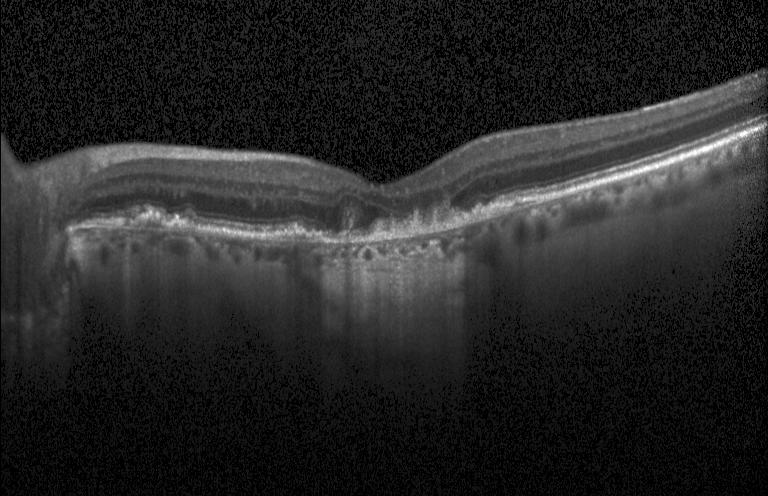
OCT line scan. Assessment: a choroidal neovascular membrane.